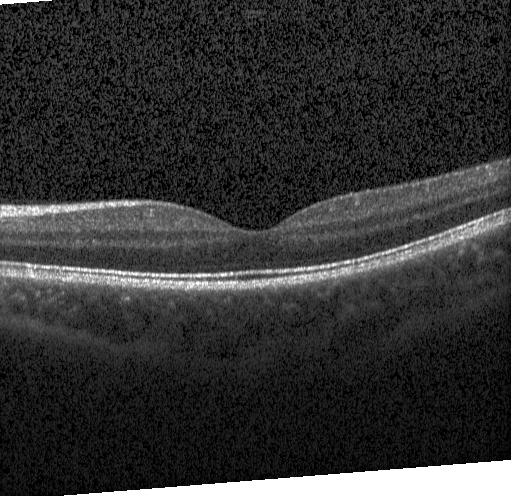

OCT B-scan — This B-scan demonstrates no evidence of choroidal neovascularization, diabetic macular edema, or drusen.